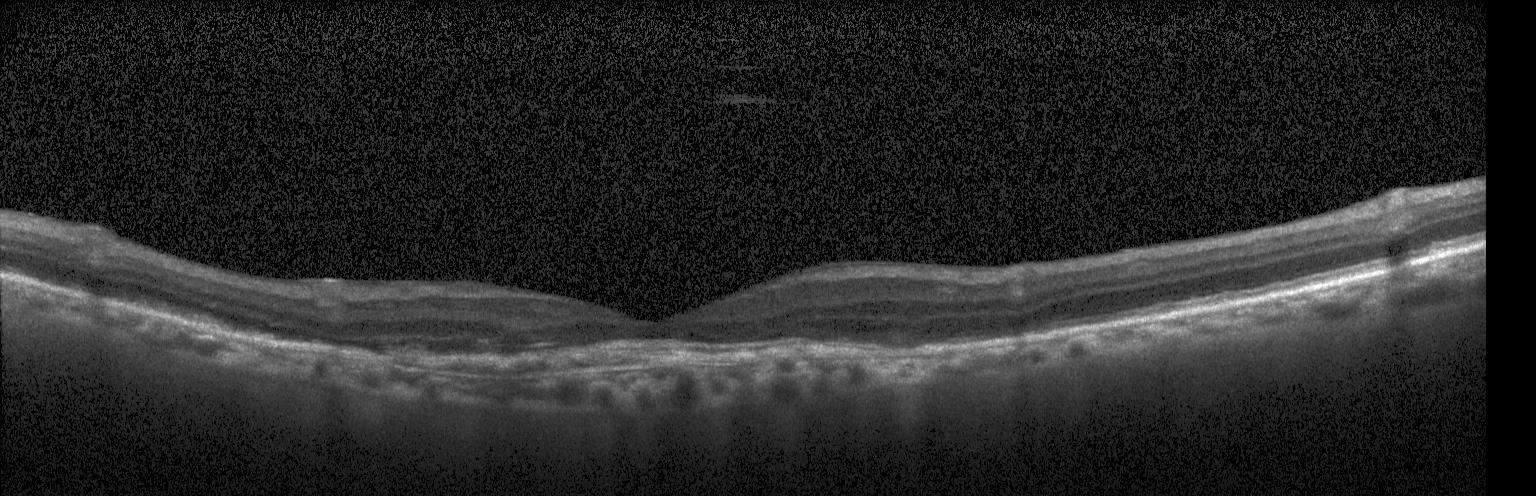 Spectral-domain OCT · acquired on a Heidelberg Spectralis · horizontal scan through the fovea · OCT line scan — A choroidal neovascular membrane.